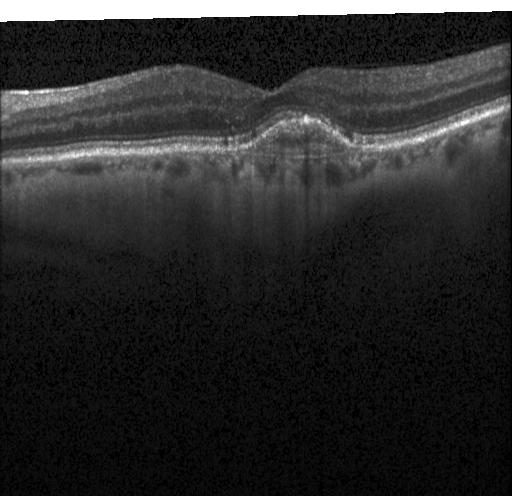

OCT scan showing a choroidal neovascular membrane.